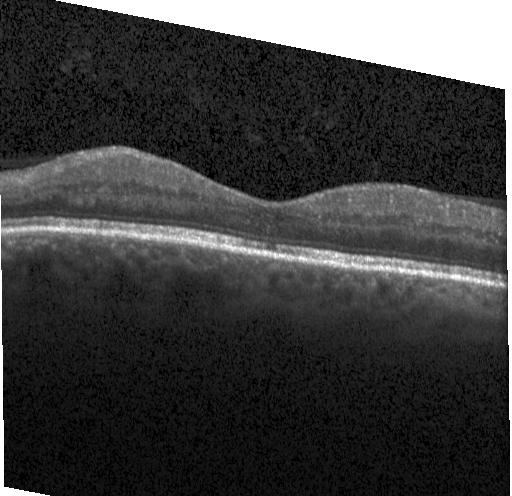

Optical coherence tomography scan; SD-OCT; instrument: Heidelberg Spectralis; fovea-centered.
Diagnosis: no choroidal neovascularization, no diabetic macular edema, and no drusen.